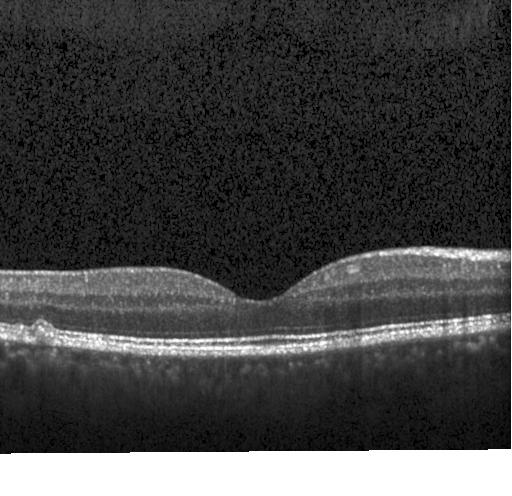 Drusen.